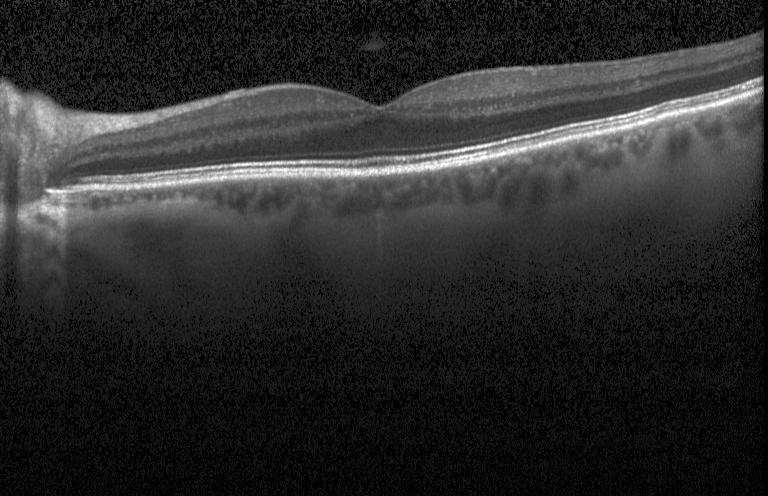

Horizontal scan through the fovea; spectral-domain OCT; Heidelberg Spectralis OCT system; OCT line scan
Finding: no evidence of choroidal neovascularization, diabetic macular edema, or drusen.